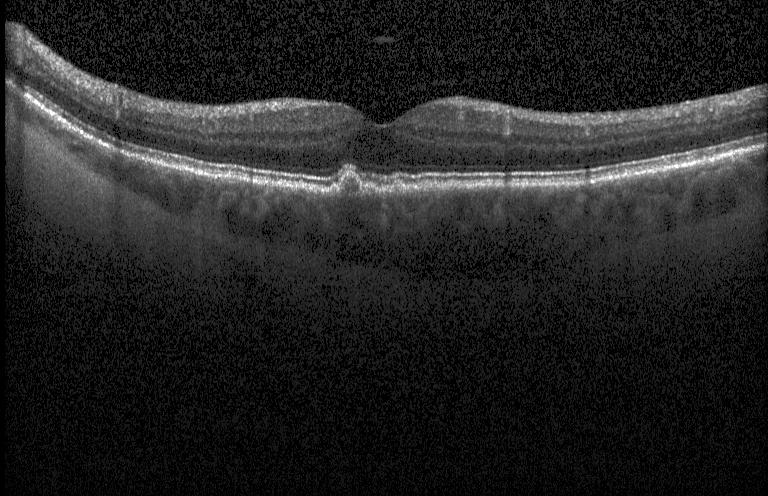

Spectral-domain OCT · Heidelberg Spectralis OCT system · optical coherence tomography B-scan
Macular OCT: multiple drusen.